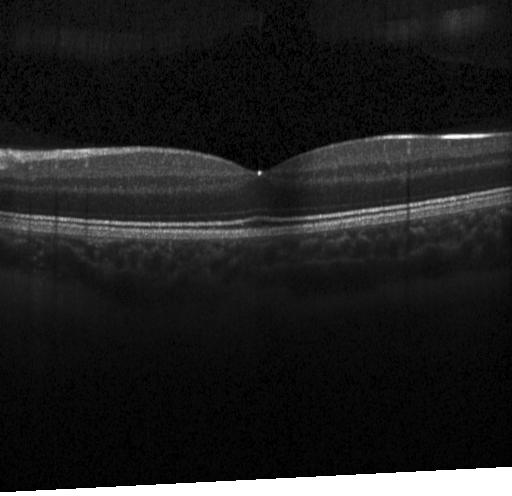
Impression: no choroidal neovascularization, diabetic macular edema, or drusen.